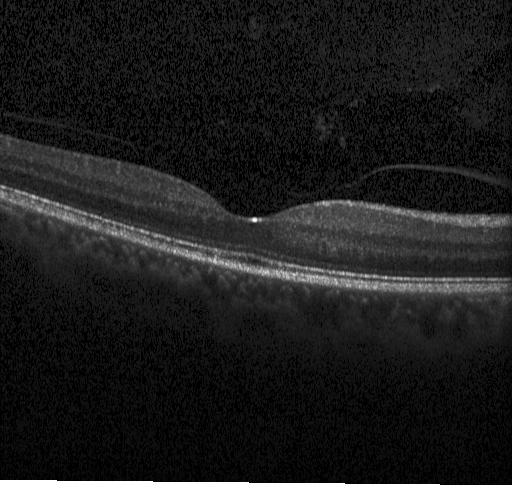
Fovea-centered · spectral-domain optical coherence tomography · retinal OCT B-scan · Heidelberg Spectralis OCT system — The scan shows no evidence of CNV, DME, or drusen.